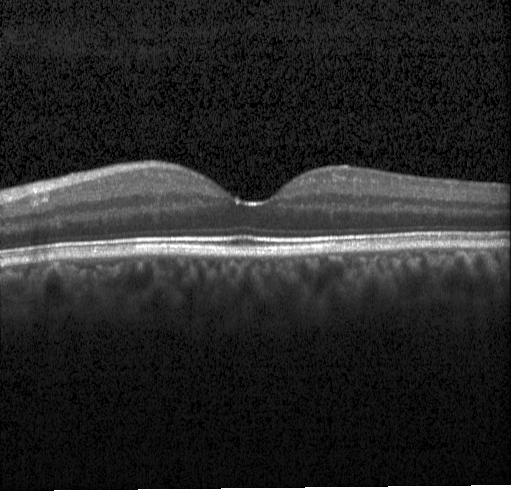
OCT finding: no choroidal neovascularization, diabetic macular edema, or drusen.